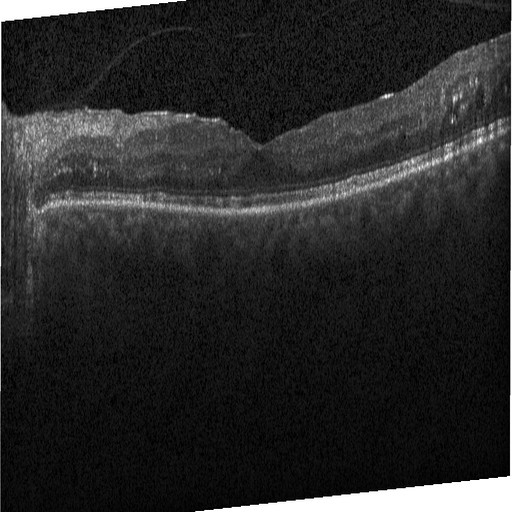
Retinal OCT cross-section showing diabetic macular edema (DME).